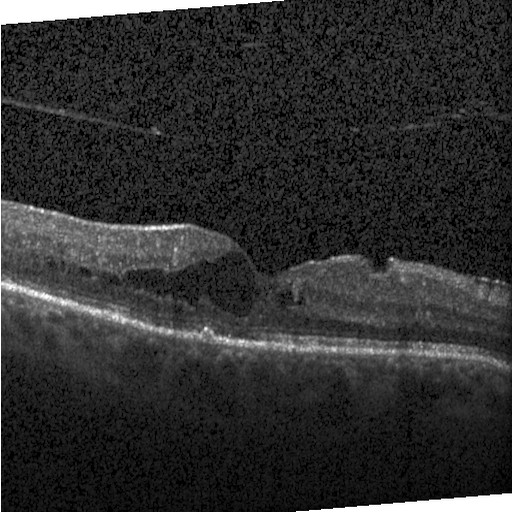 OCT line scan. Diabetic macular edema (DME).